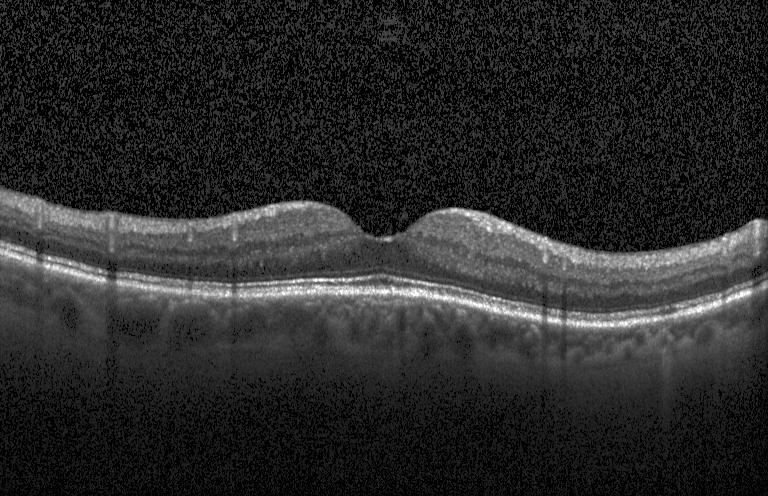

Instrument: Heidelberg Spectralis. OCT B-scan — This B-scan demonstrates neither choroidal neovascularization, diabetic macular edema, nor drusen.